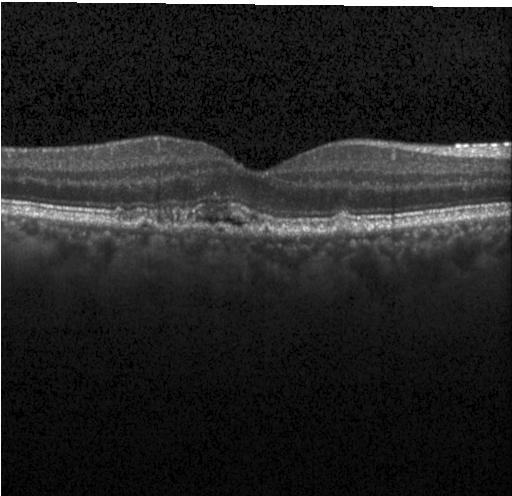 Through the macula · retinal OCT cross-section · instrument: Heidelberg Spectralis.
Finding: a choroidal neovascular membrane.